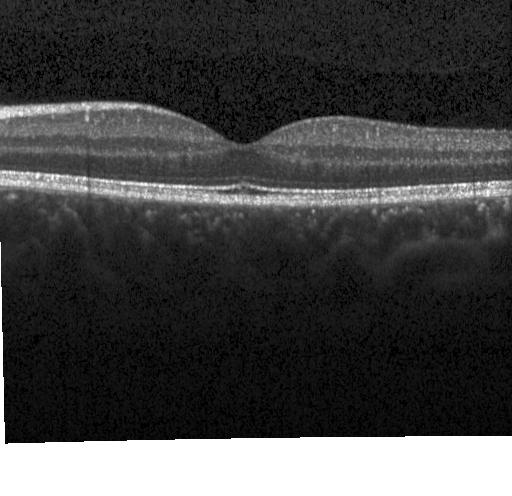 Optical coherence tomography scan · centered on the fovea
Finding: no choroidal neovascularization, no diabetic macular edema, and no drusen.